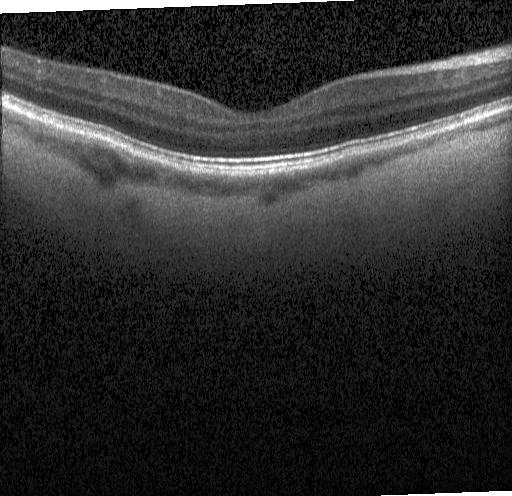
Heidelberg Spectralis; retinal OCT B-scan; horizontal scan through the fovea. The scan shows no CNV, no DME, and no drusen.